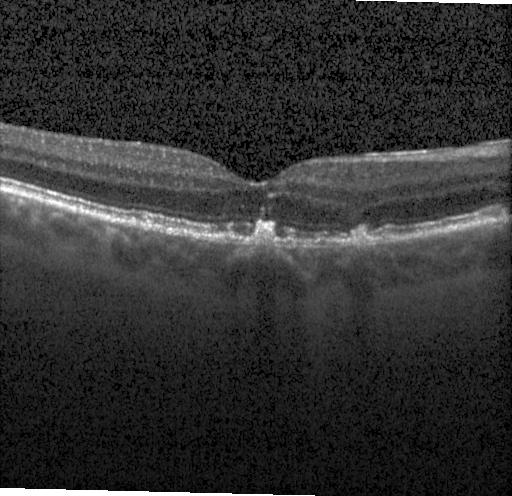

Through the macula, instrument: Heidelberg Spectralis, OCT B-scan, SD-OCT
Macular OCT: a choroidal neovascular membrane.